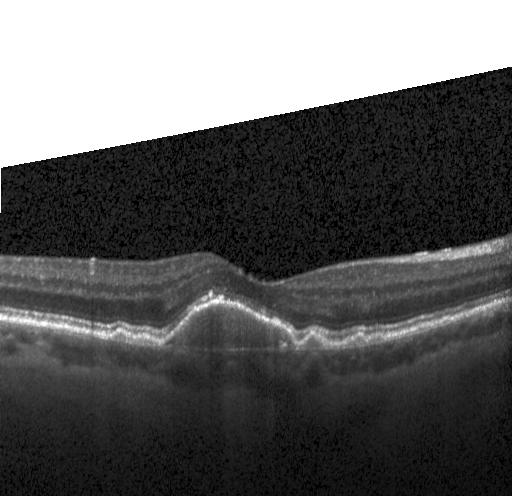

Optical coherence tomography B-scan. SD-OCT. Heidelberg Spectralis. Assessment: a choroidal neovascular membrane.